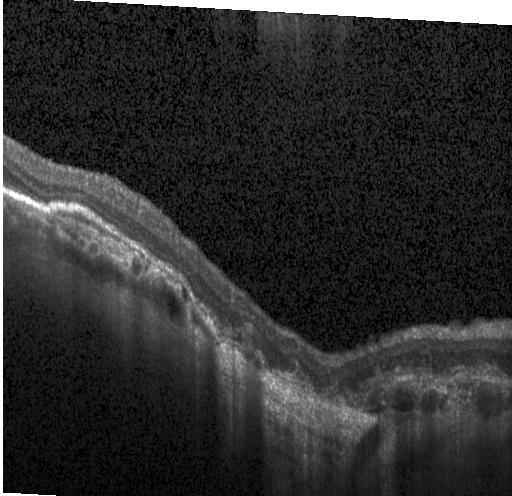 Macular OCT demonstrating a choroidal neovascular membrane.